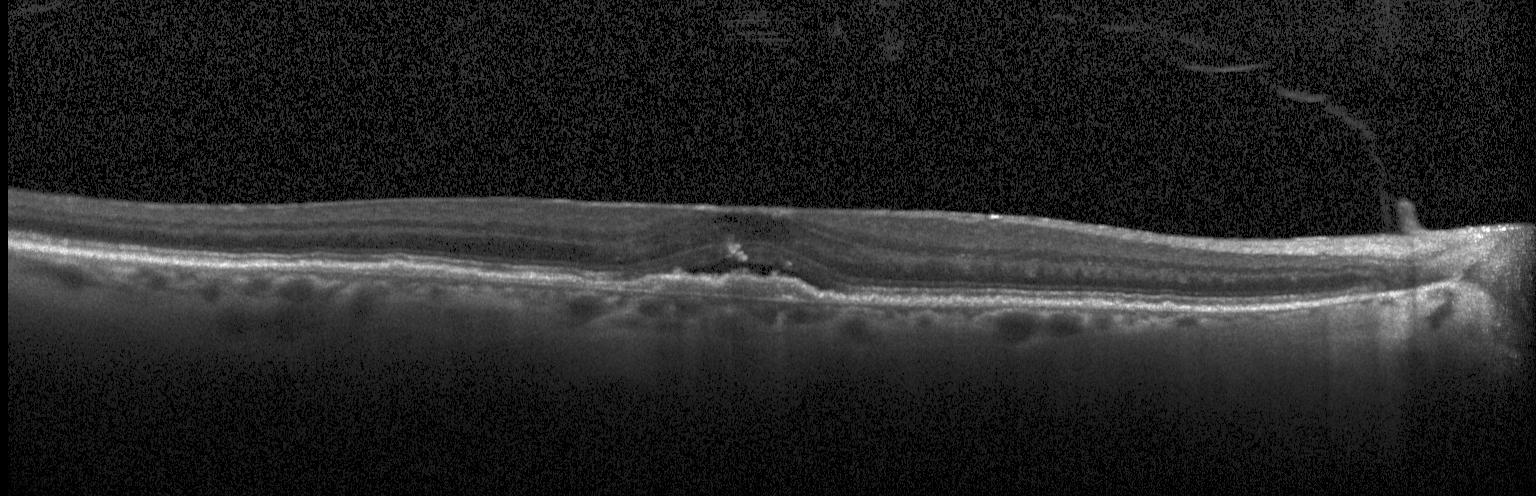
Retinal OCT cross-section
Finding: choroidal neovascularization.